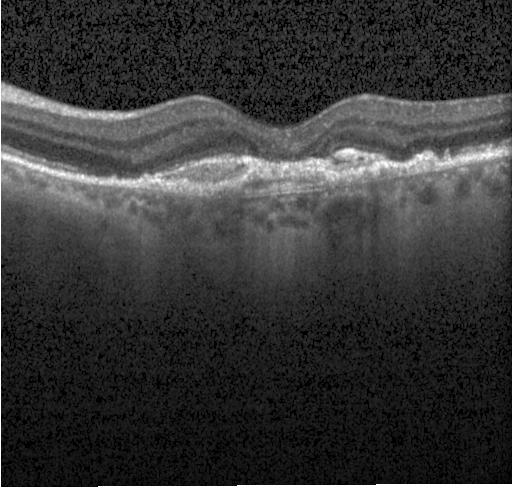

Macular scan, spectral-domain optical coherence tomography, optical coherence tomography scan. Macular OCT: a choroidal neovascular membrane.